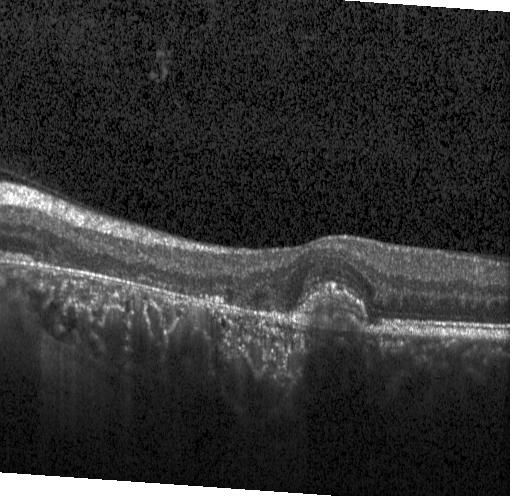
Horizontal scan through the fovea · optical coherence tomography scan · acquired on a Heidelberg Spectralis — Finding: a choroidal neovascular membrane.